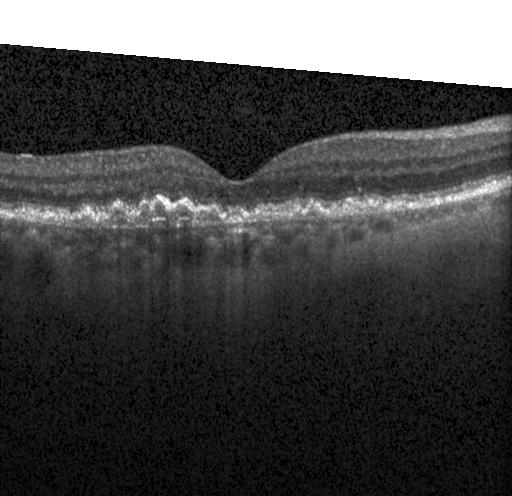

Acquired on a Heidelberg Spectralis · SD-OCT · OCT B-scan · horizontal scan through the fovea
Dx: choroidal neovascularization (CNV).